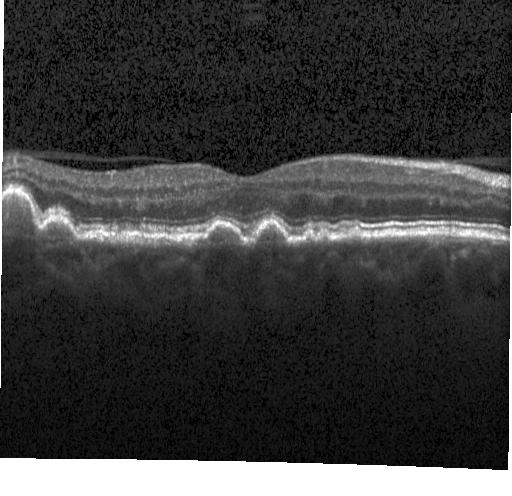
Macular scan · instrument: Heidelberg Spectralis · retinal OCT cross-section — This B-scan demonstrates sub-RPE drusenoid deposits.